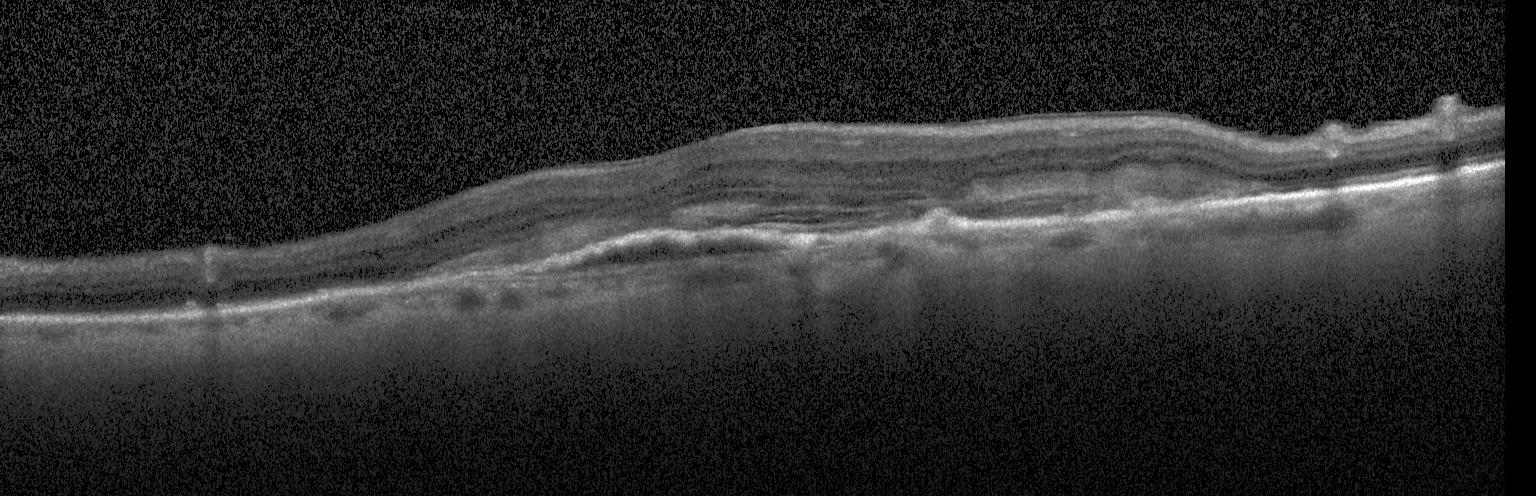
Instrument: Heidelberg Spectralis · optical coherence tomography scan.
Assessment: a choroidal neovascular membrane.